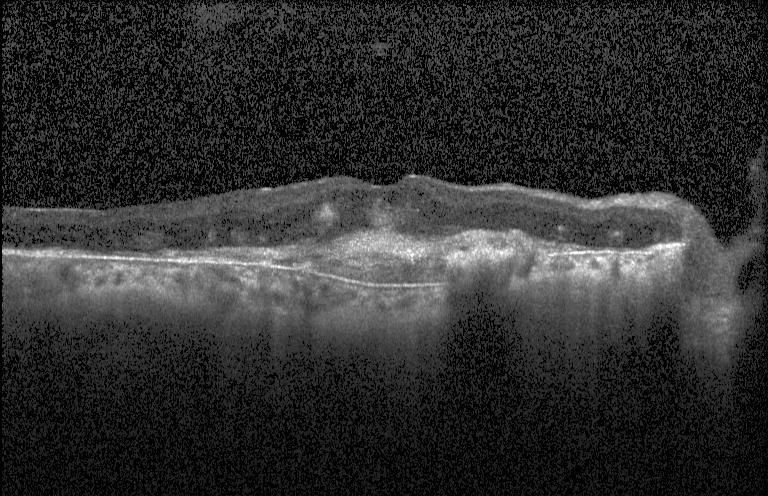

Acquired on a Heidelberg Spectralis; OCT B-scan. Impression: choroidal neovascularization (CNV).